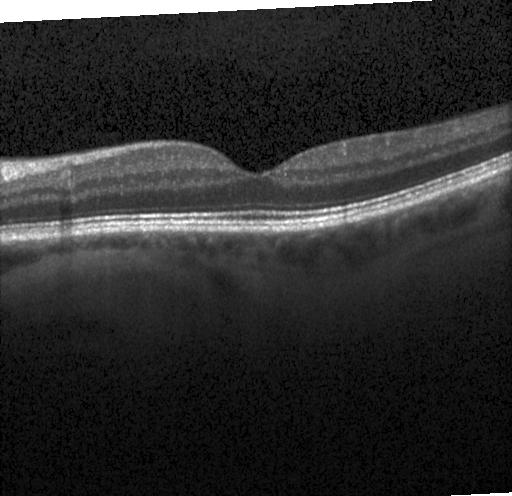
OCT B-scan
This B-scan demonstrates no choroidal neovascularization, diabetic macular edema, or drusen.